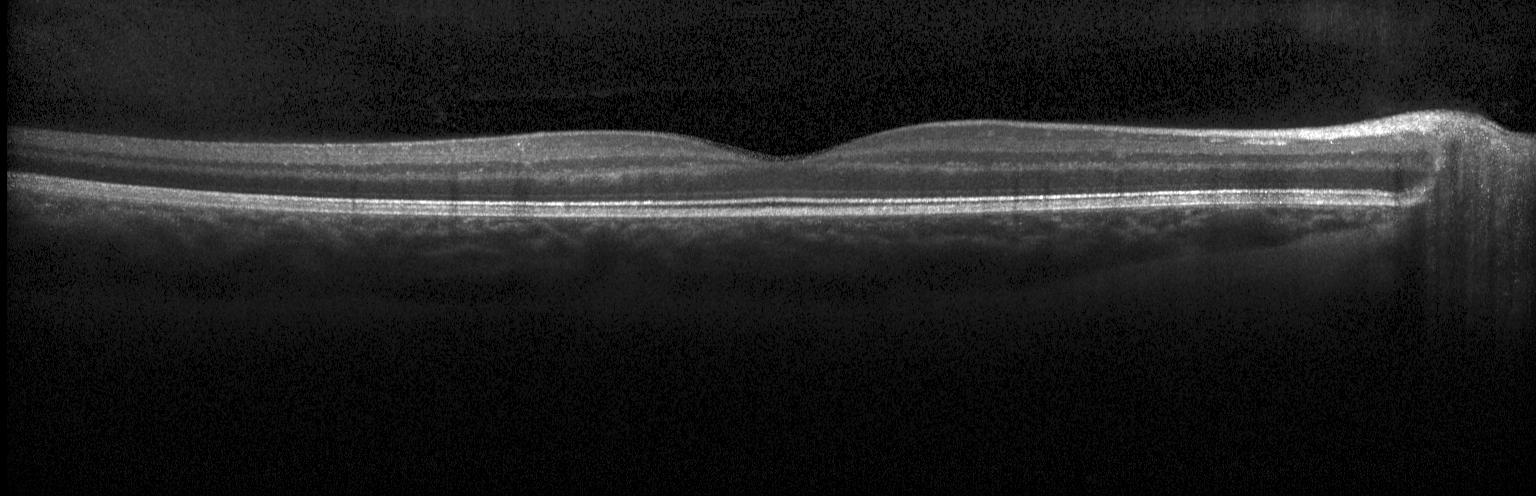

Acquired on a Heidelberg Spectralis; optical coherence tomography scan; horizontal scan through the fovea; SD-OCT. The scan shows no choroidal neovascularization, diabetic macular edema, or drusen.